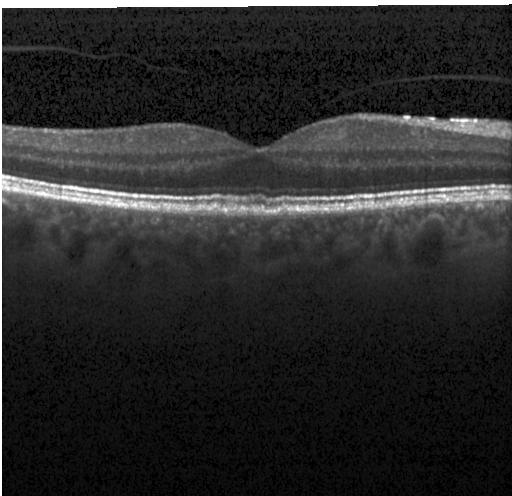
Diagnosis: multiple drusen.